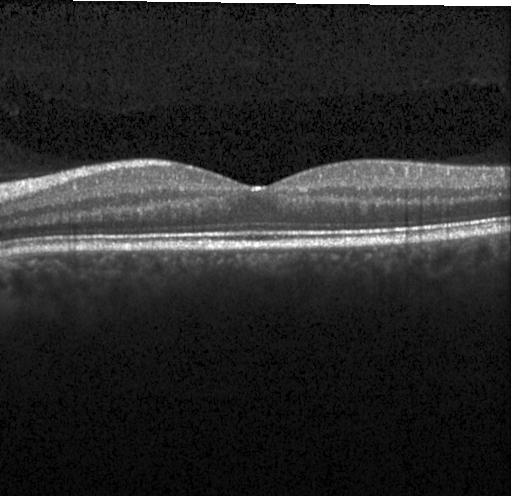 OCT line scan. Impression: no CNV, no DME, and no drusen.